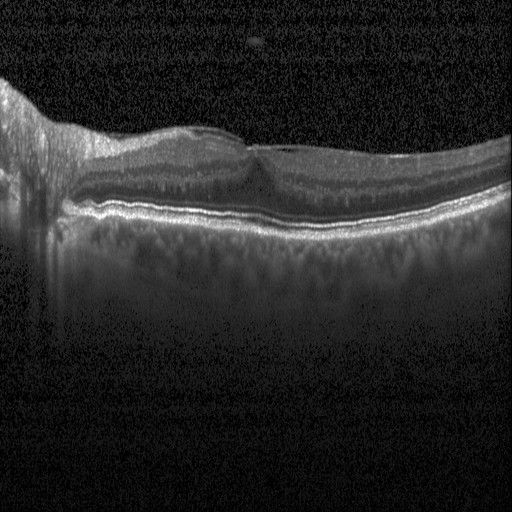
Heidelberg Spectralis; OCT line scan; centered on the fovea; SD-OCT. Diagnosis: DME.